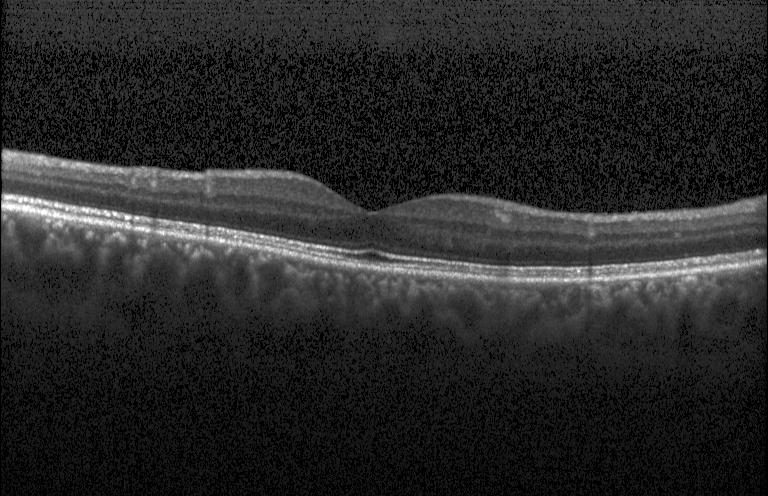 Spectral-domain optical coherence tomography, through the macula, optical coherence tomography scan — Assessment: no CNV, DME, or drusen.